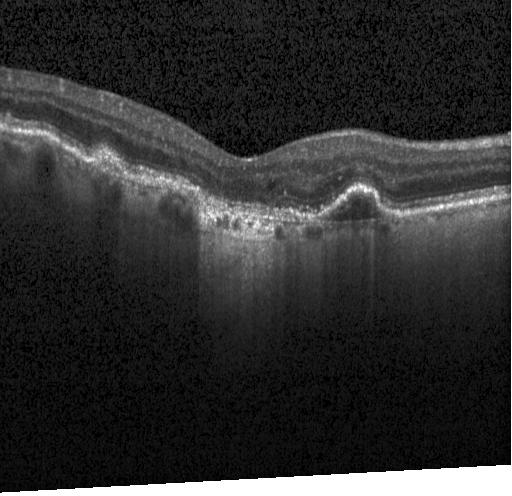 Spectral-domain optical coherence tomography. Fovea-centered. Heidelberg Spectralis. Retinal OCT B-scan.
Diagnosis: choroidal neovascularization (CNV).